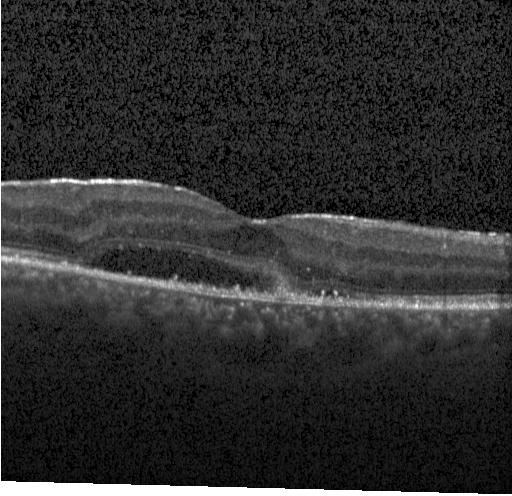

Choroidal neovascularization (CNV).